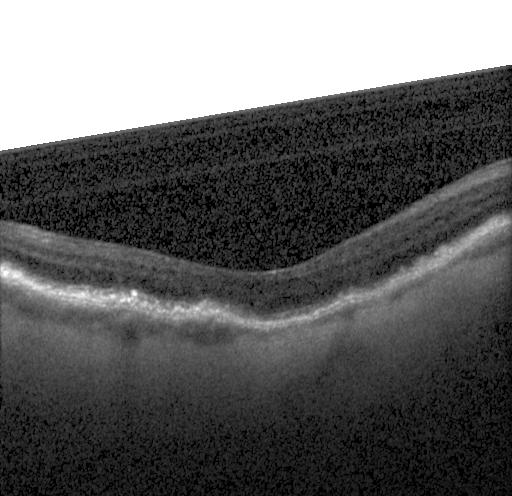
Optical coherence tomography B-scan. Instrument: Heidelberg Spectralis. Through the macula.
Impression: a choroidal neovascular membrane.